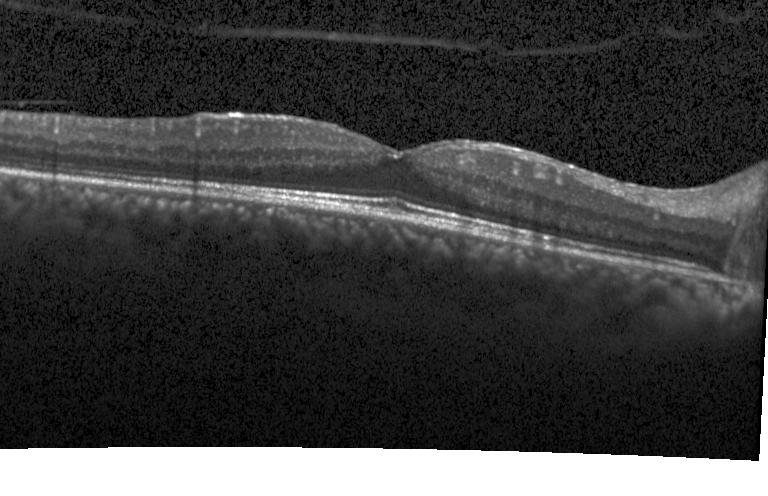 OCT B-scan. Impression: neither choroidal neovascularization, diabetic macular edema, nor drusen.